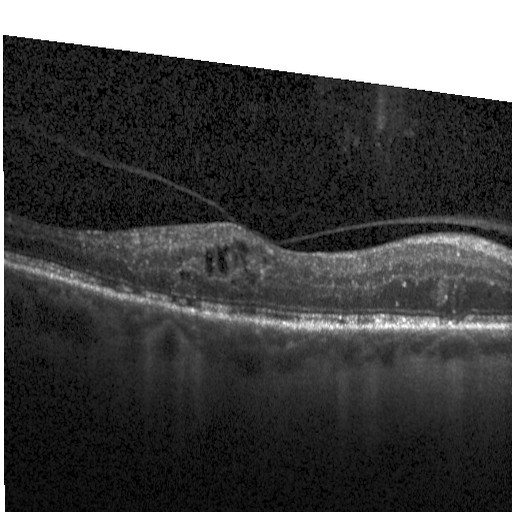

Macular OCT: diabetic macular edema (DME).